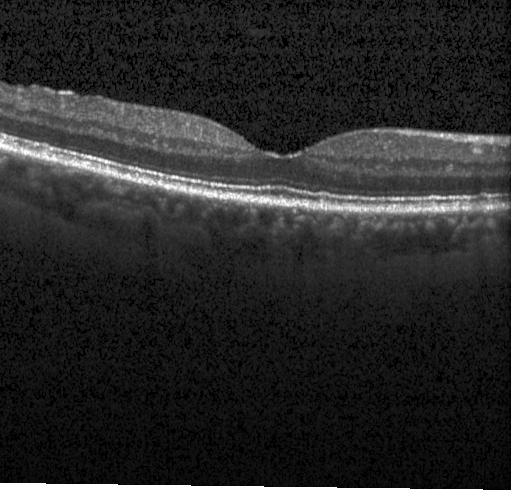
Through the macula; retinal OCT B-scan — Diagnosis: no evidence of choroidal neovascularization, diabetic macular edema, or drusen.